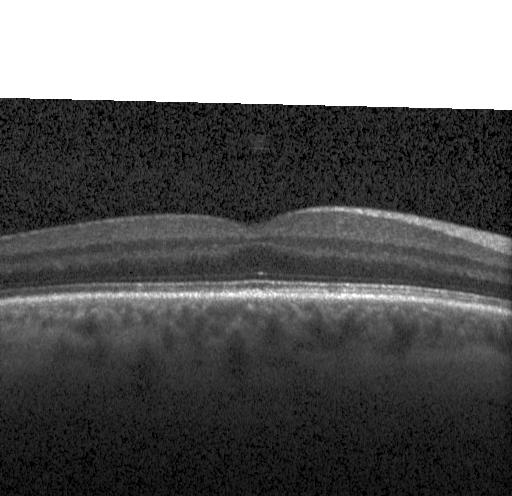

OCT B-scan. Centered on the fovea. Heidelberg Spectralis. Finding: no evidence of choroidal neovascularization, diabetic macular edema, or drusen.